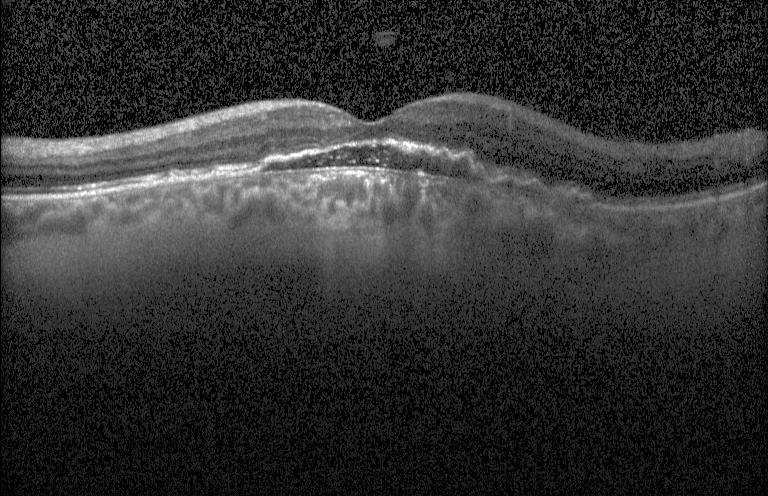
Horizontal scan through the fovea. Instrument: Heidelberg Spectralis. Retinal OCT cross-section. Spectral-domain optical coherence tomography — Assessment: a choroidal neovascular membrane.